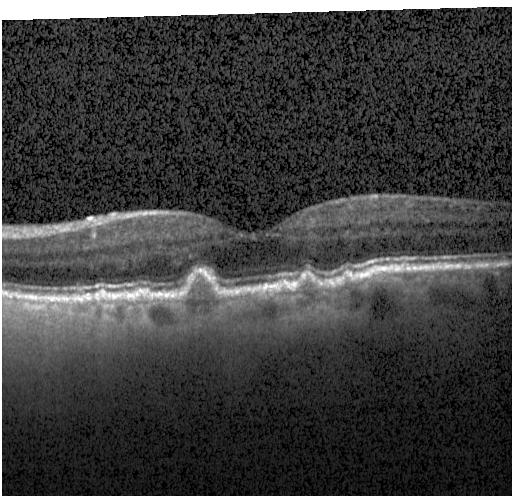

Optical coherence tomography B-scan. This B-scan demonstrates drusen.